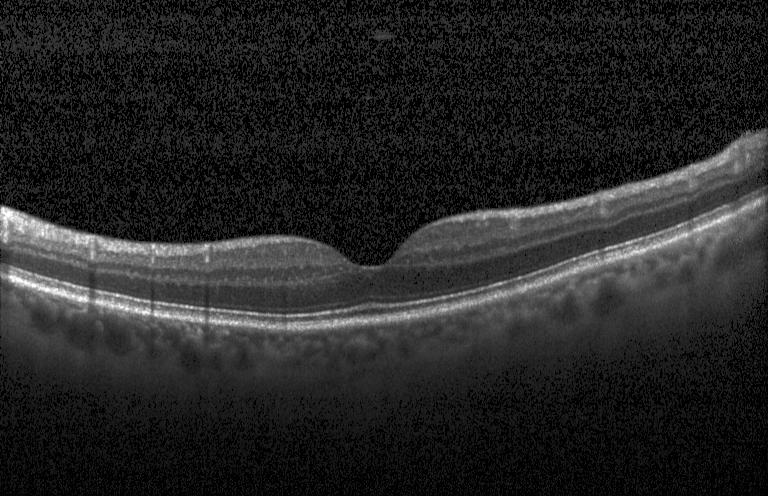
Diagnosis: no choroidal neovascularization, diabetic macular edema, or drusen.